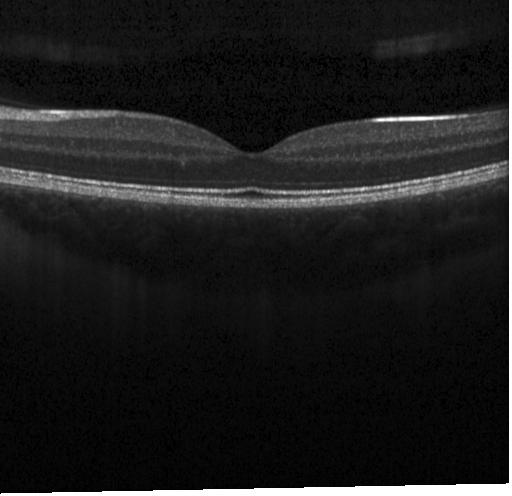 Retinal OCT B-scan
OCT finding: no evidence of CNV, DME, or drusen.